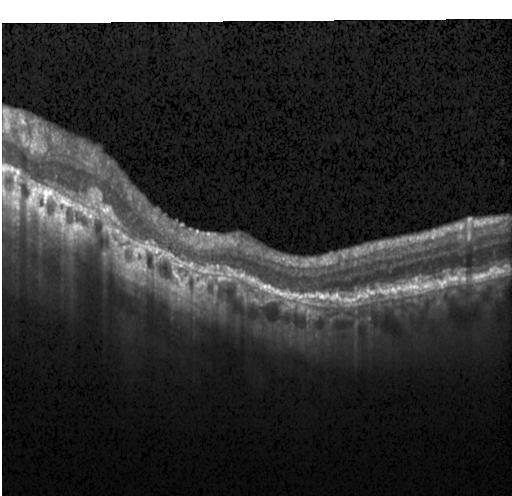 Optical coherence tomography scan
OCT finding: CNV.